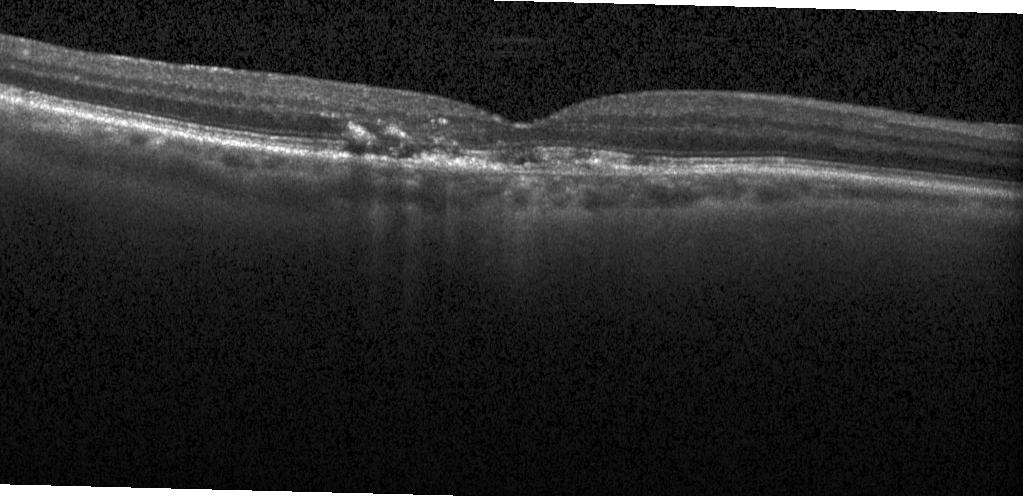
SD-OCT, OCT line scan — CNV.